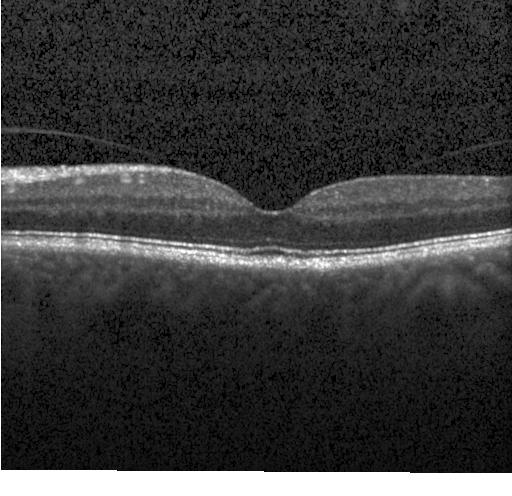 Finding: no CNV, no DME, and no drusen.